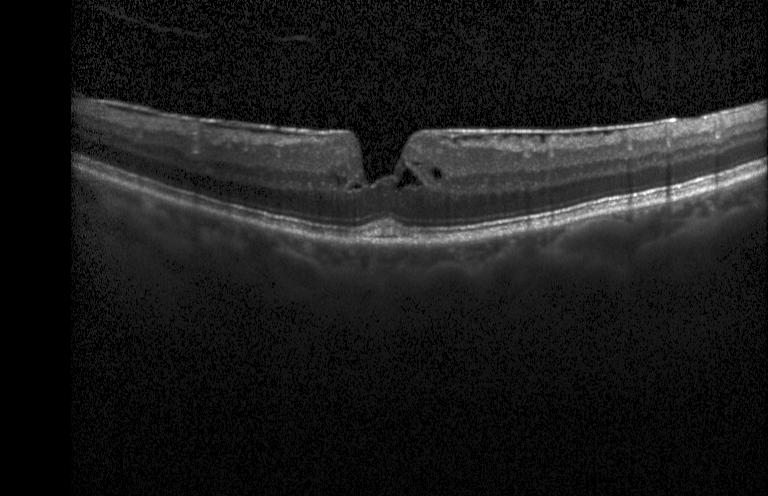

Spectral-domain optical coherence tomography. Macular scan. Heidelberg Spectralis OCT system. Retinal OCT B-scan — Dx: diabetic macular edema (DME).